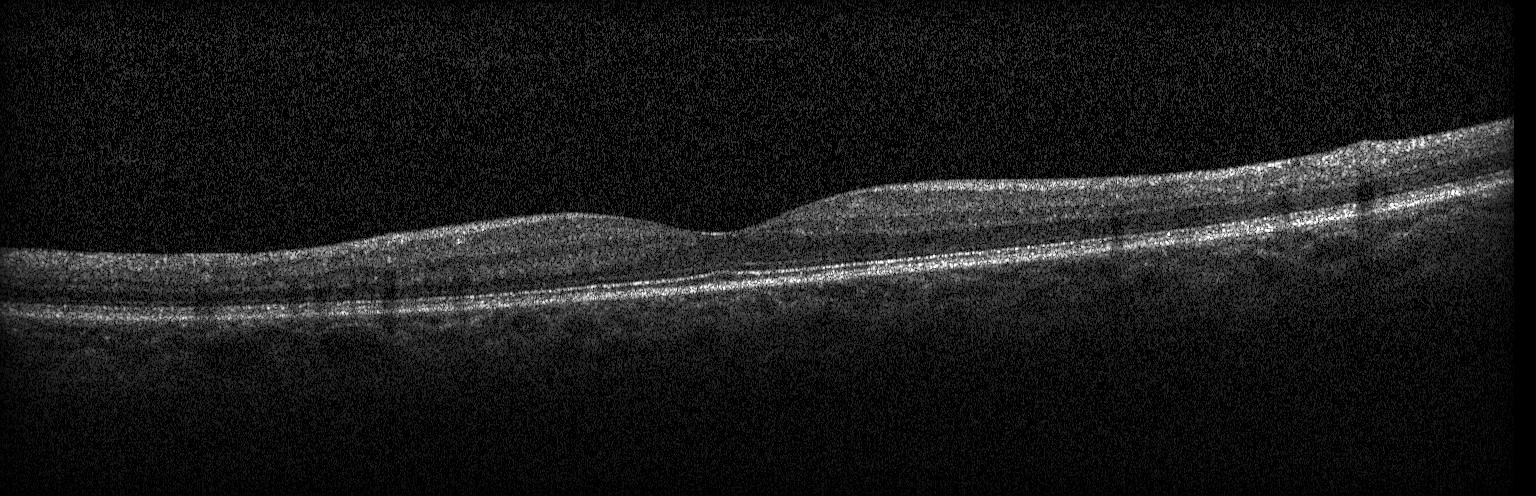

Dx: neither CNV, DME, nor drusen.